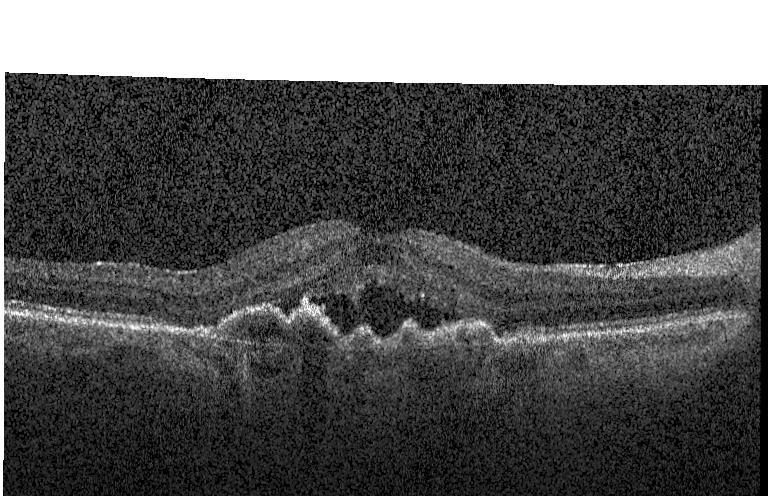 A choroidal neovascular membrane.